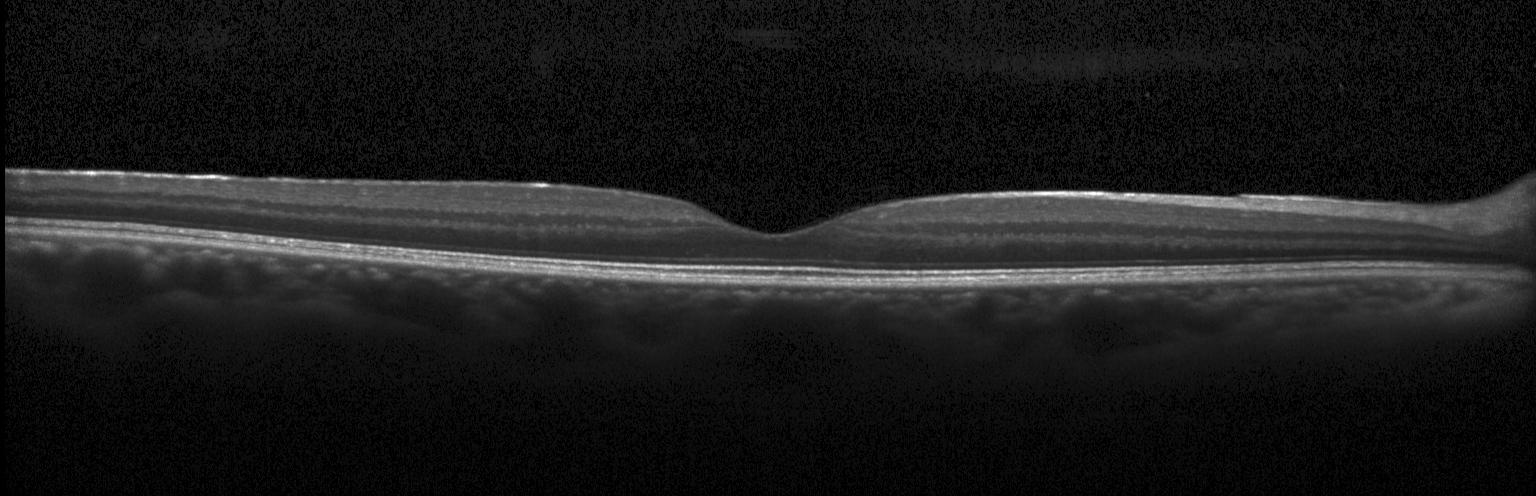

Retinal OCT B-scan
Impression: no evidence of CNV, DME, or drusen.